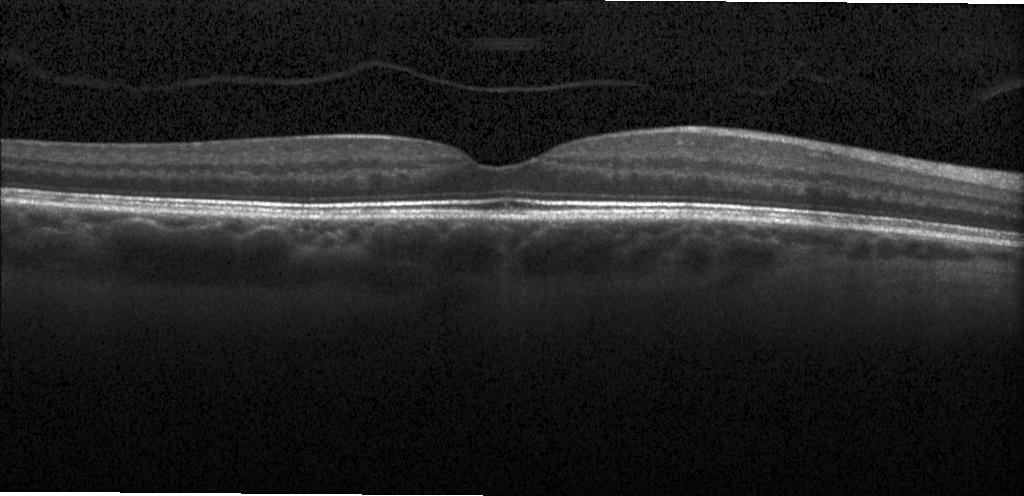
Dx: no choroidal neovascularization, diabetic macular edema, or drusen.